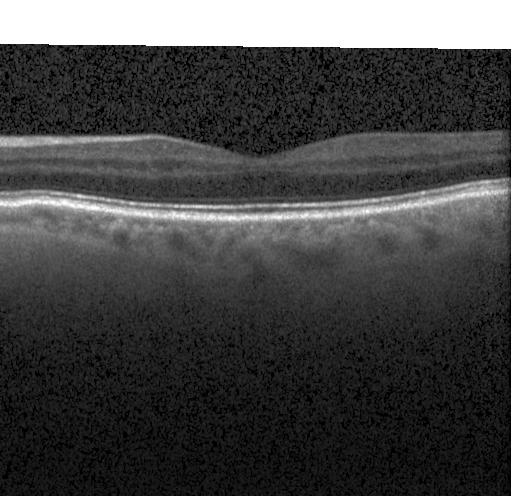
Centered on the fovea, OCT line scan, Heidelberg Spectralis.
Assessment: no choroidal neovascularization, diabetic macular edema, or drusen.